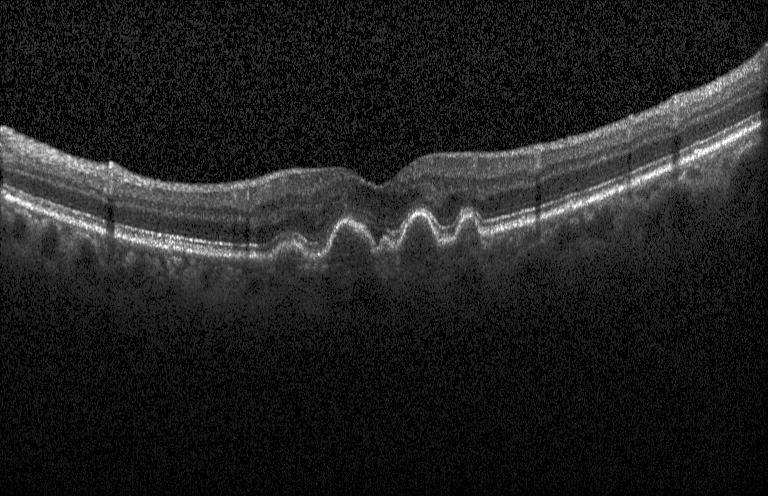

Retinal OCT cross-section showing multiple drusen.